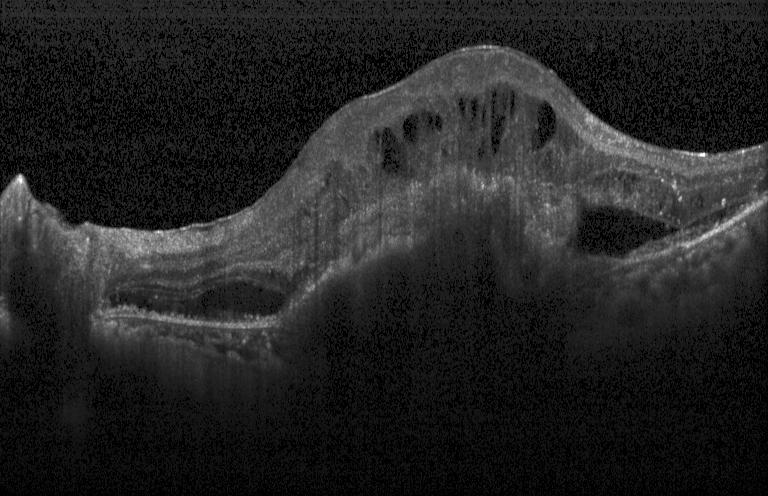
Heidelberg Spectralis OCT system. Retinal OCT B-scan. Fovea-centered. Spectral-domain OCT — Finding: CNV.